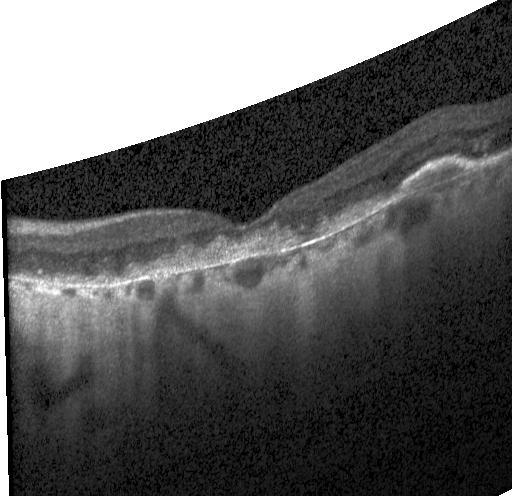
Impression: a choroidal neovascular membrane.